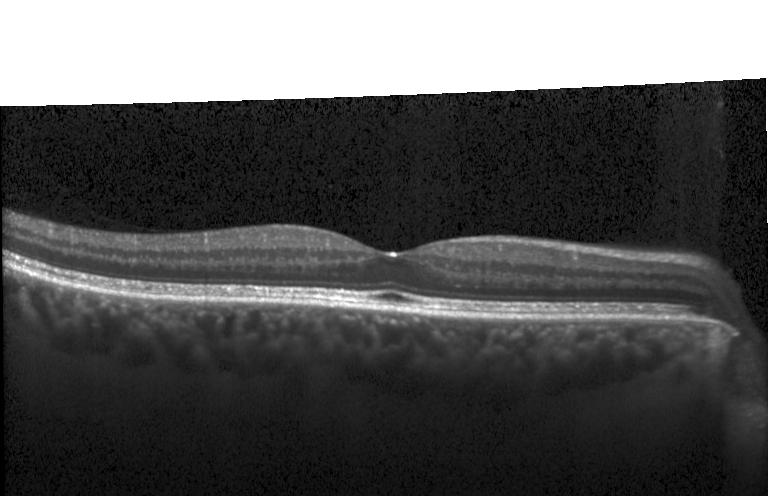 Retinal OCT cross-section. Macular OCT: no evidence of choroidal neovascularization, diabetic macular edema, or drusen.